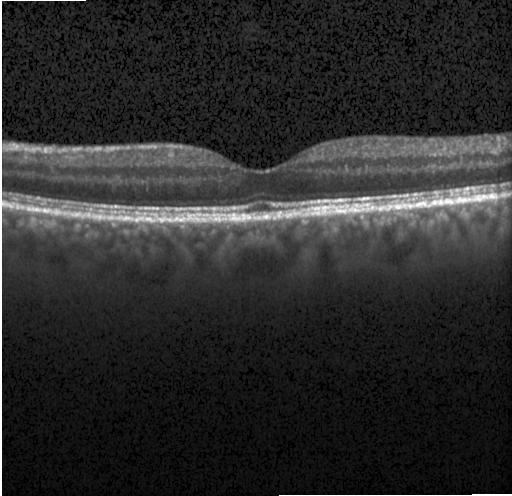
Instrument: Heidelberg Spectralis, OCT line scan
Macular OCT: neither choroidal neovascularization, diabetic macular edema, nor drusen.